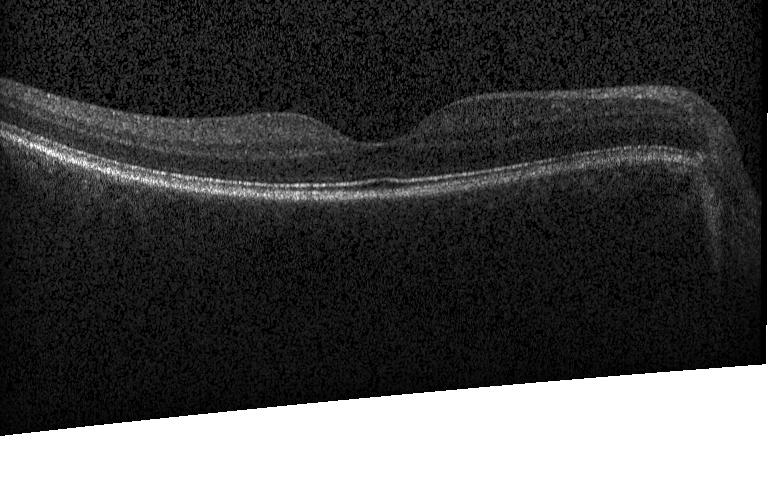 This B-scan demonstrates no choroidal neovascularization, no diabetic macular edema, and no drusen.